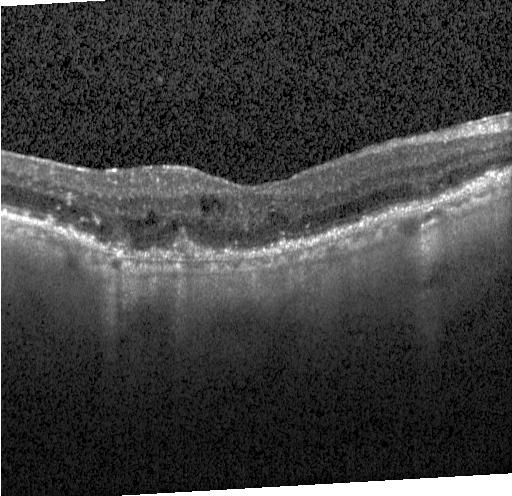
Instrument: Heidelberg Spectralis, fovea-centered, optical coherence tomography B-scan
Assessment: CNV.